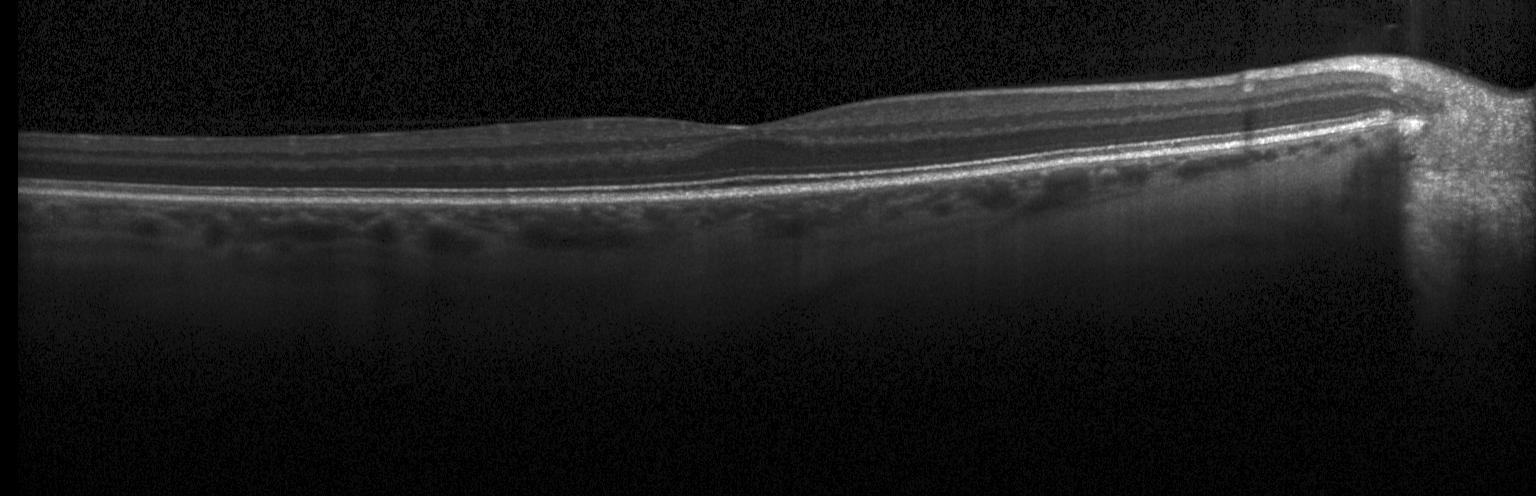
Optical coherence tomography scan; fovea-centered — Diagnosis: neither CNV, DME, nor drusen.